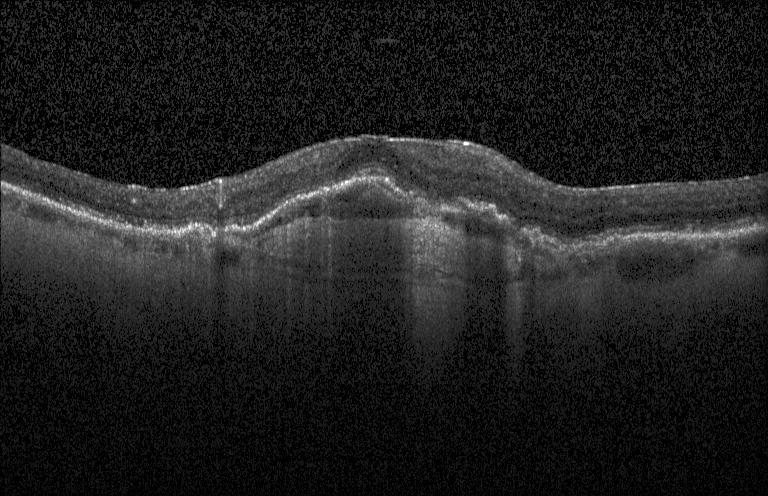

Dx: a choroidal neovascular membrane.